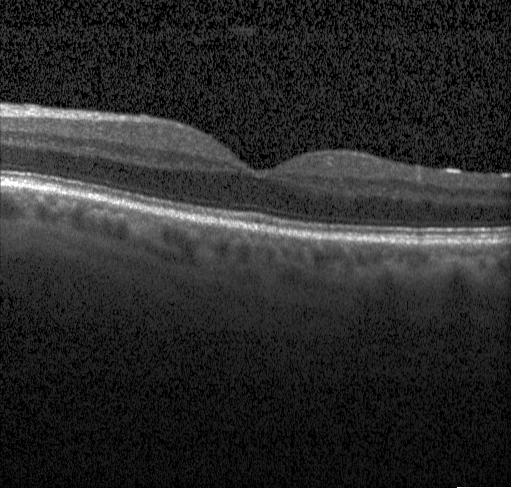

OCT B-scan
This B-scan demonstrates no evidence of choroidal neovascularization, diabetic macular edema, or drusen.